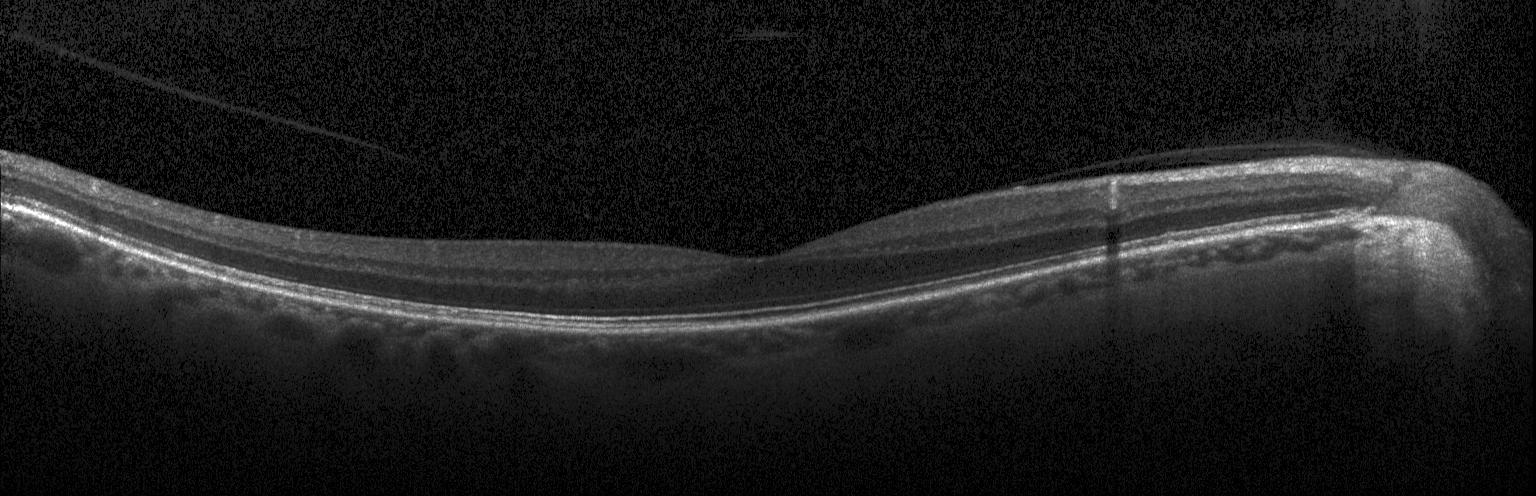

Finding: no choroidal neovascularization, diabetic macular edema, or drusen.